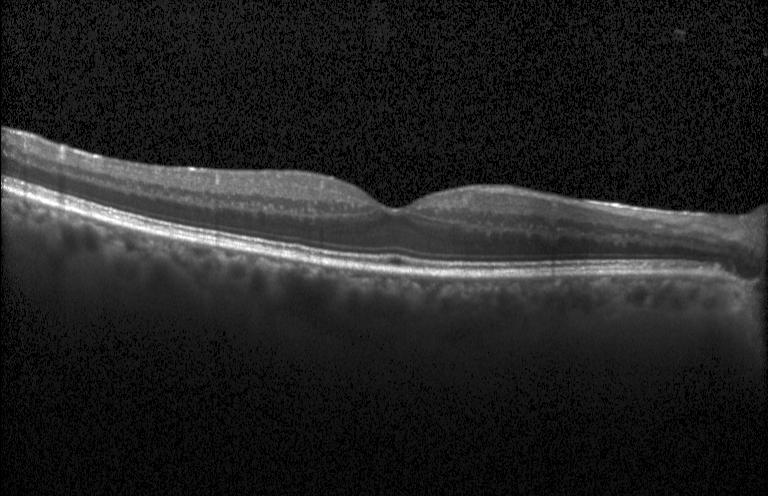

Diagnosis: neither choroidal neovascularization, diabetic macular edema, nor drusen.